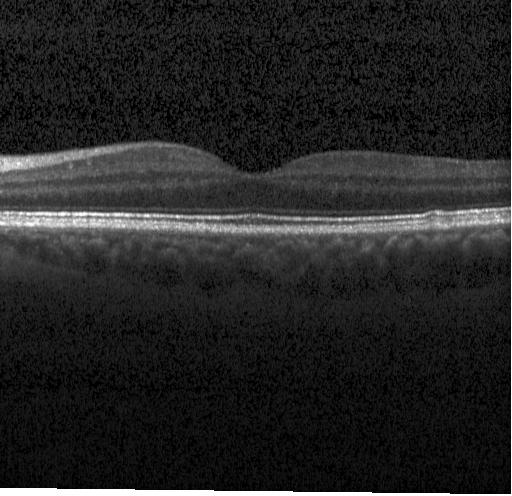
Optical coherence tomography scan. Diagnosis: no evidence of CNV, DME, or drusen.